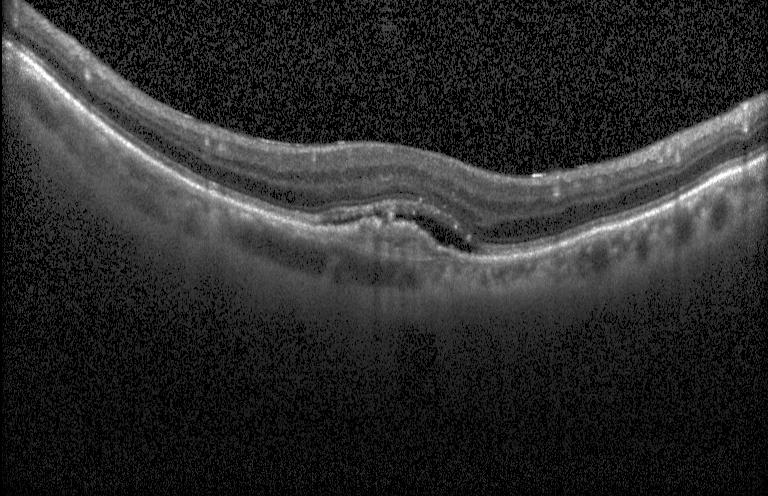 Spectral-domain OCT, OCT line scan, fovea-centered, acquired on a Heidelberg Spectralis. The scan shows a choroidal neovascular membrane.